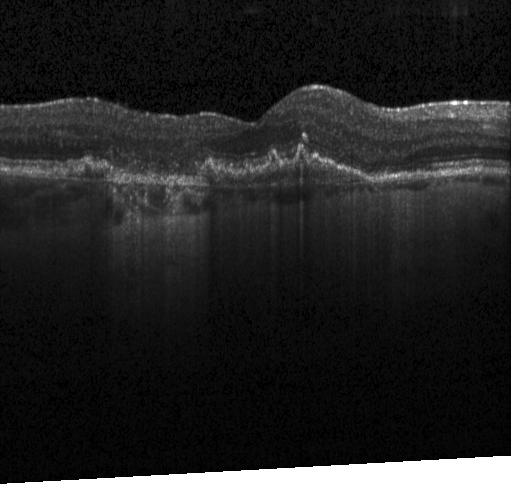
Retinal OCT B-scan; spectral-domain OCT; Heidelberg Spectralis OCT system; centered on the fovea.
Finding: a choroidal neovascular membrane.